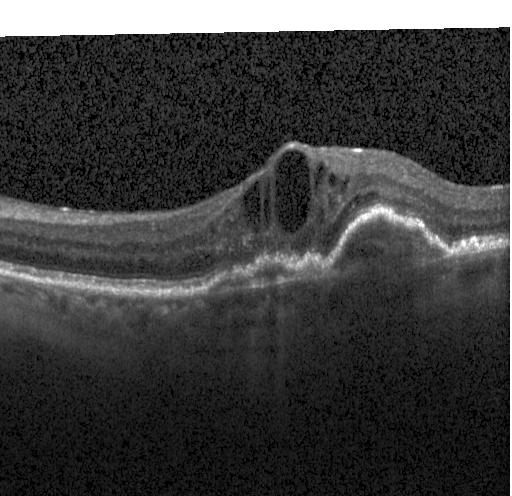

Spectral-domain optical coherence tomography. Optical coherence tomography B-scan. Acquired on a Heidelberg Spectralis. Through the macula.
Impression: choroidal neovascularization.